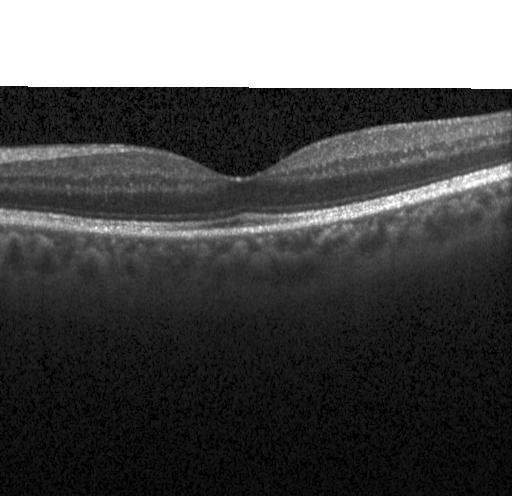
Acquired on a Heidelberg Spectralis · spectral-domain OCT · OCT B-scan · through the macula — Assessment: neither choroidal neovascularization, diabetic macular edema, nor drusen.